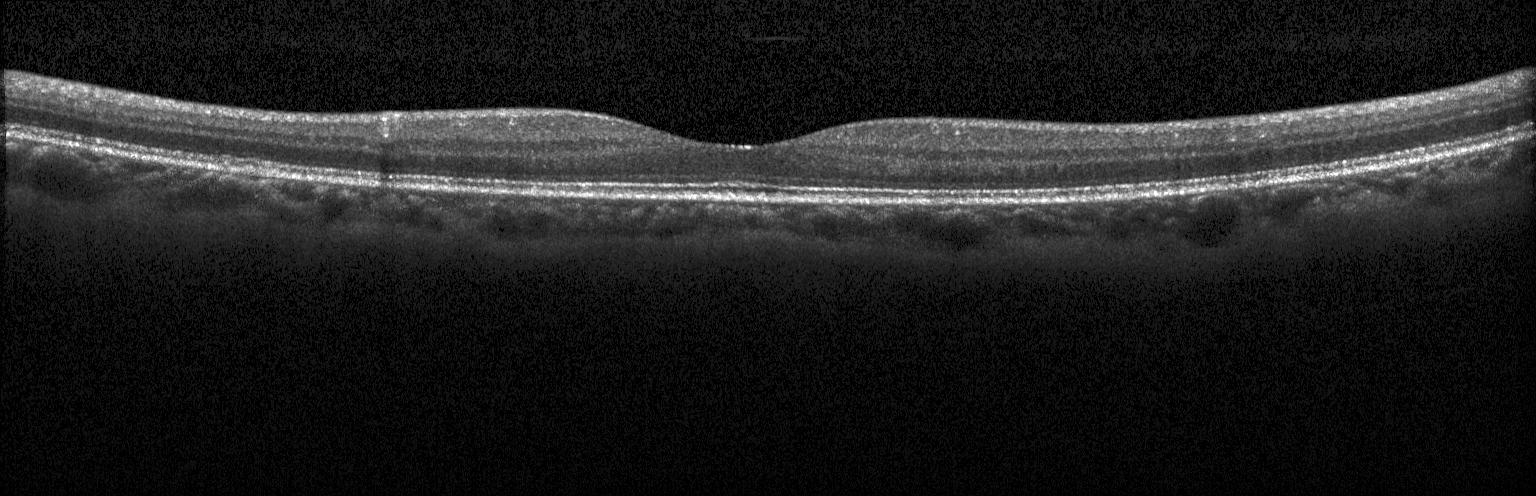
Retinal OCT B-scan; spectral-domain optical coherence tomography; through the macula — Impression: no choroidal neovascularization, diabetic macular edema, or drusen.